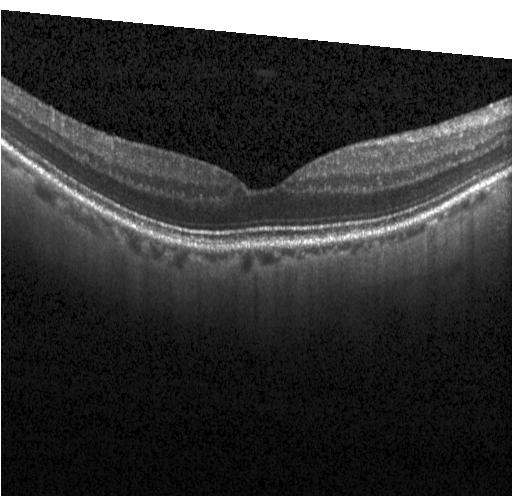 Centered on the fovea. OCT B-scan. Spectral-domain optical coherence tomography. Heidelberg Spectralis OCT system
Finding: no choroidal neovascularization, no diabetic macular edema, and no drusen.